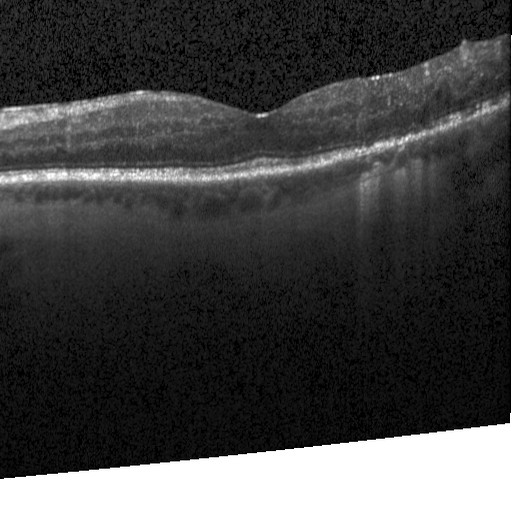

Optical coherence tomography scan. Heidelberg Spectralis. Spectral-domain OCT
Impression: DME.